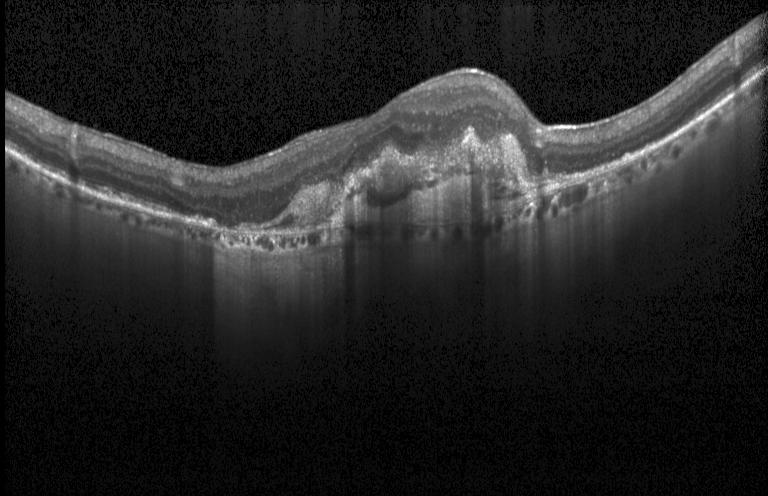 Spectral-domain optical coherence tomography, Heidelberg Spectralis, centered on the fovea, OCT B-scan. Finding: a choroidal neovascular membrane.